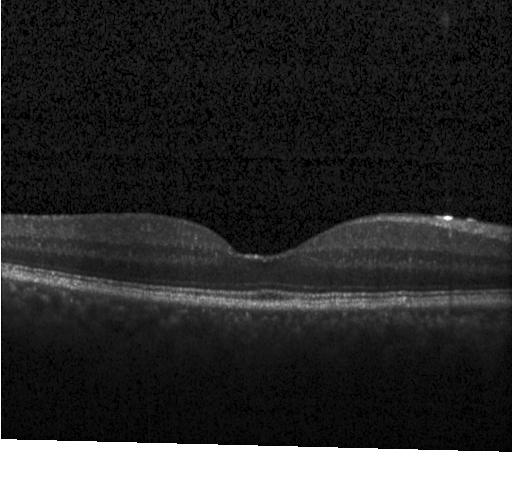

Macular OCT demonstrating no CNV, DME, or drusen.